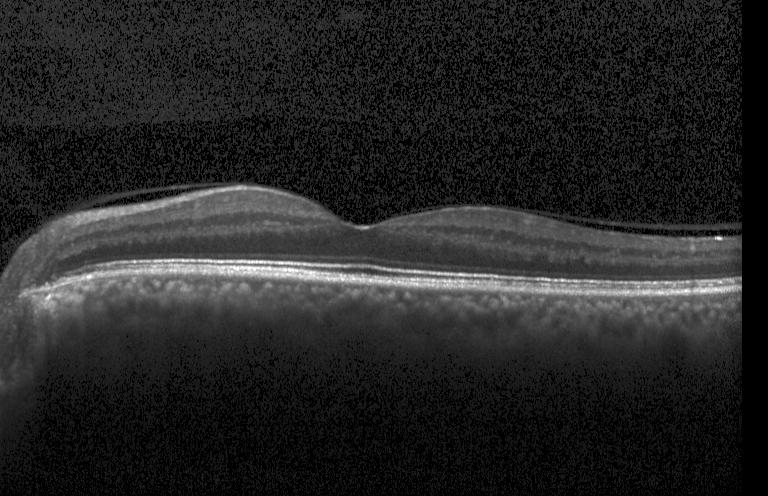
Diagnosis: neither choroidal neovascularization, diabetic macular edema, nor drusen.